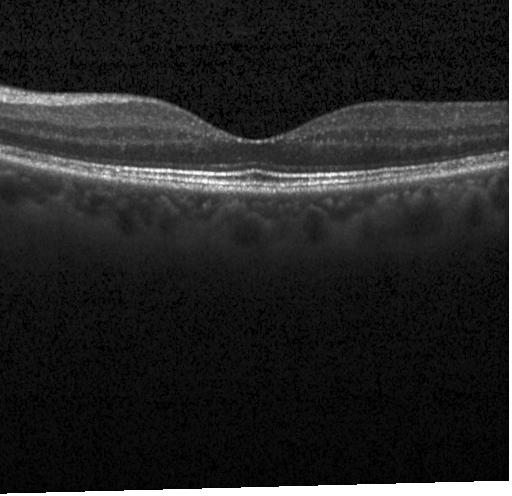

Macular OCT: no CNV, DME, or drusen.